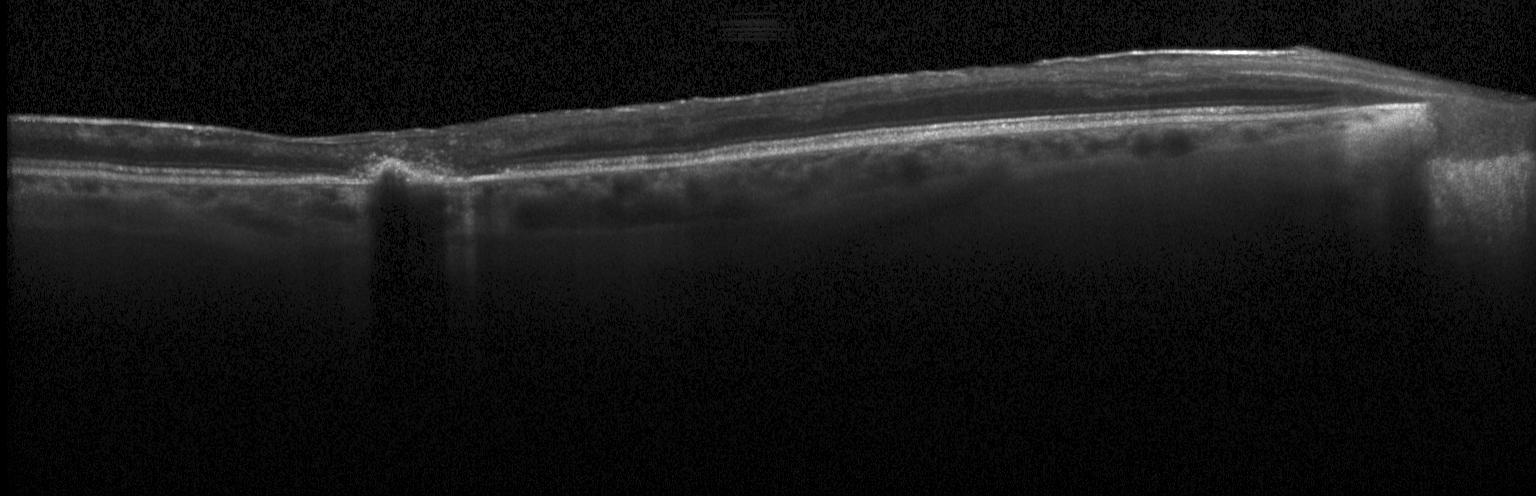

Optical coherence tomography B-scan · instrument: Heidelberg Spectralis · SD-OCT.
Diagnosis: CNV.